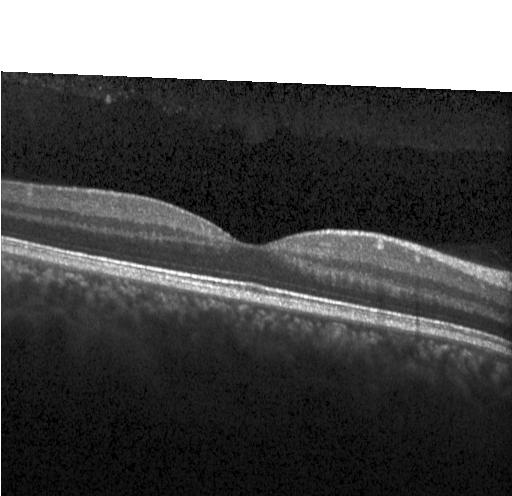
Retinal OCT cross-section — Assessment: no choroidal neovascularization, diabetic macular edema, or drusen.